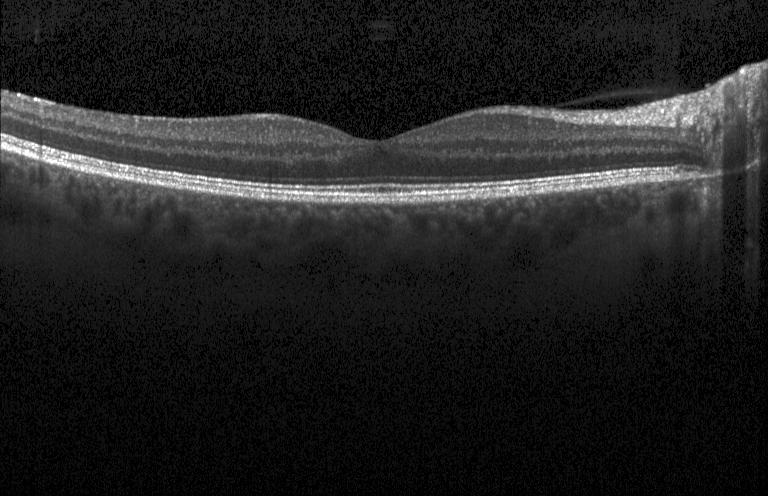
SD-OCT. Retinal OCT cross-section. Acquired on a Heidelberg Spectralis. Macular scan — Diagnosis: no CNV, DME, or drusen.